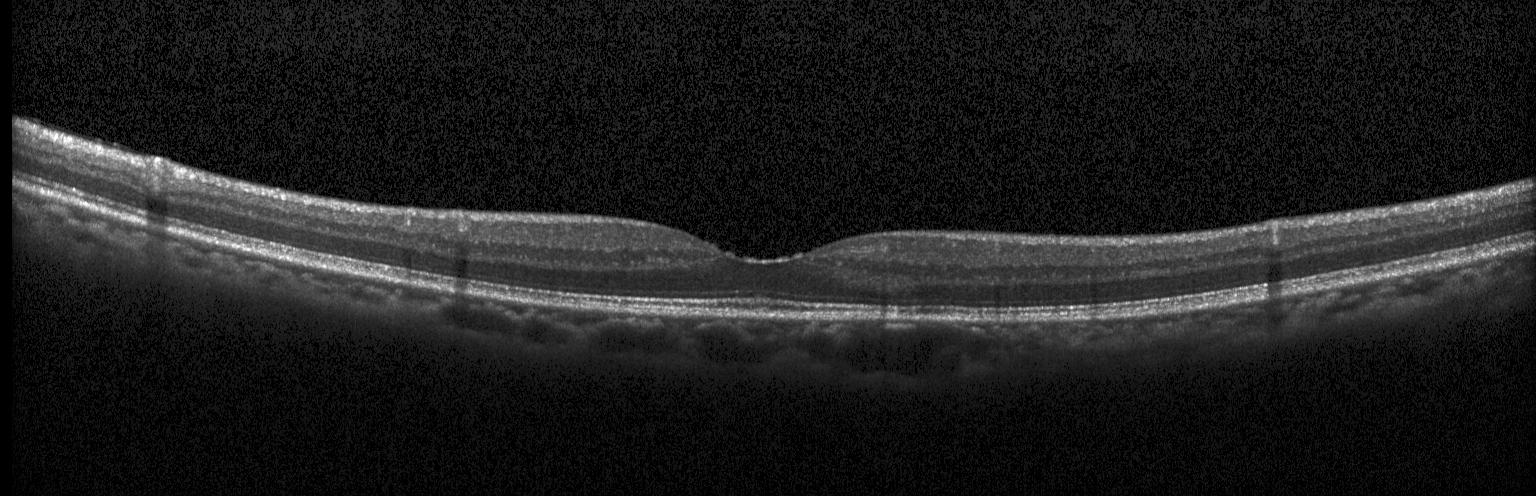 Spectral-domain OCT B-scan: neither choroidal neovascularization, diabetic macular edema, nor drusen.